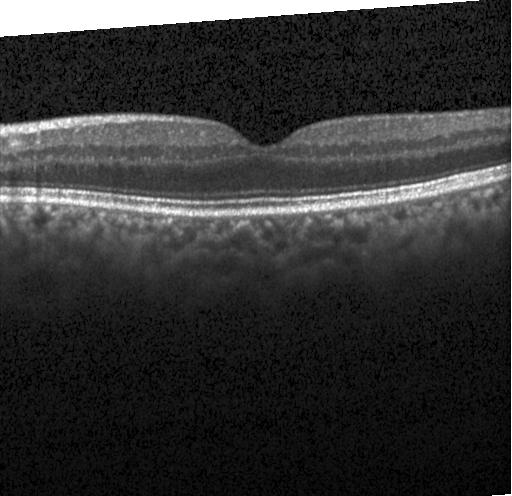 Optical coherence tomography scan; SD-OCT; Heidelberg Spectralis OCT system.
Assessment: neither choroidal neovascularization, diabetic macular edema, nor drusen.